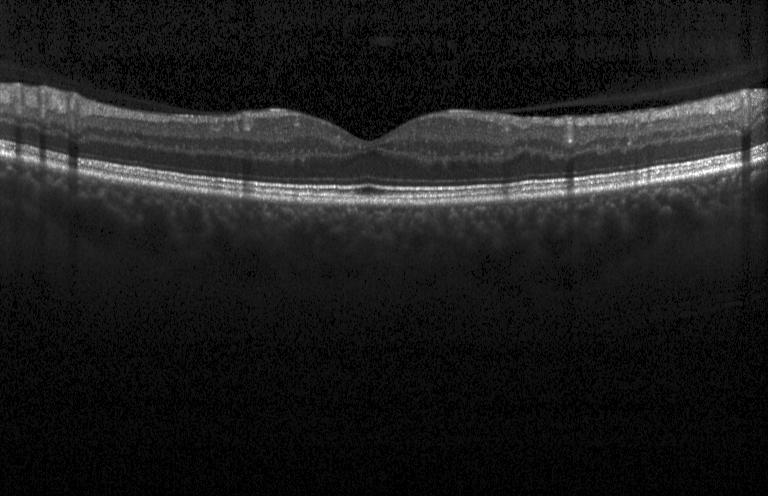 Macular OCT demonstrating no evidence of choroidal neovascularization, diabetic macular edema, or drusen.